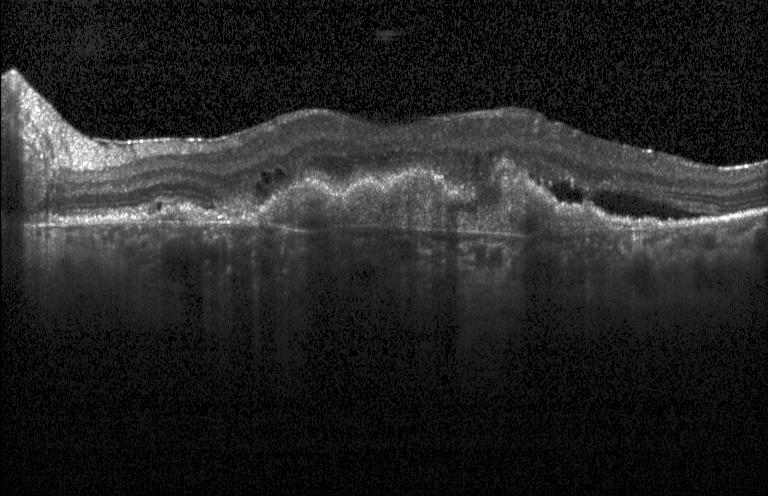

Retinal OCT cross-section
Macular OCT: a choroidal neovascular membrane.